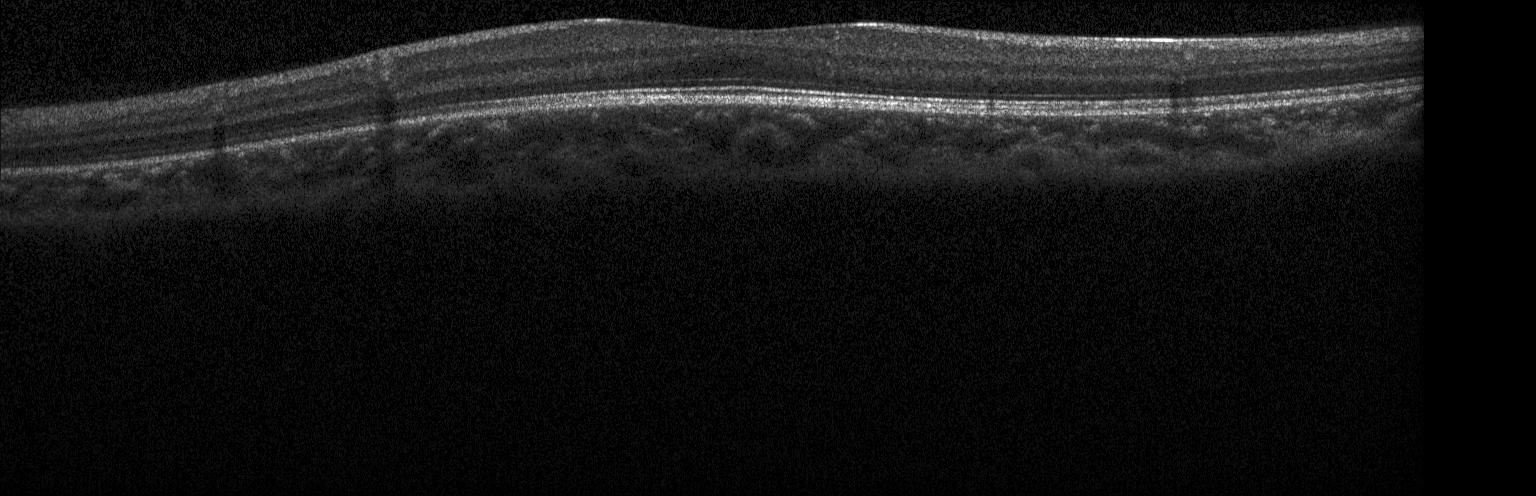

Retinal OCT B-scan. Spectral-domain optical coherence tomography. Fovea-centered. Heidelberg Spectralis OCT system
This B-scan demonstrates no choroidal neovascularization, diabetic macular edema, or drusen.